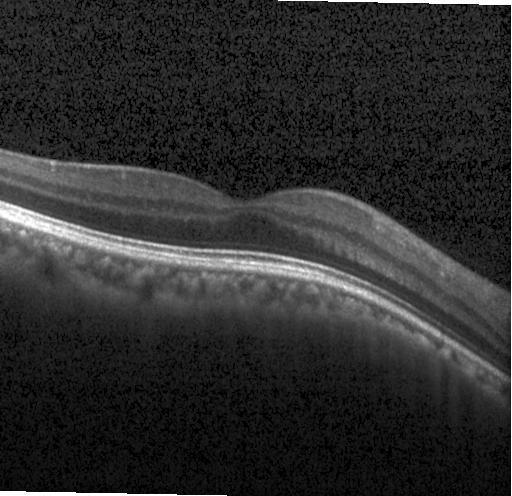

Optical coherence tomography B-scan; spectral-domain OCT. The scan shows no CNV, DME, or drusen.